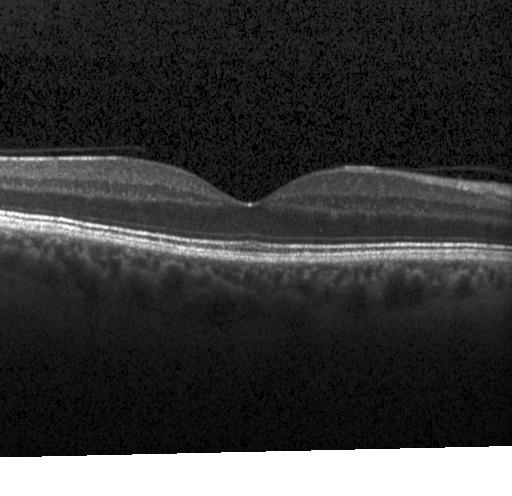
Diagnosis: no choroidal neovascularization, no diabetic macular edema, and no drusen.